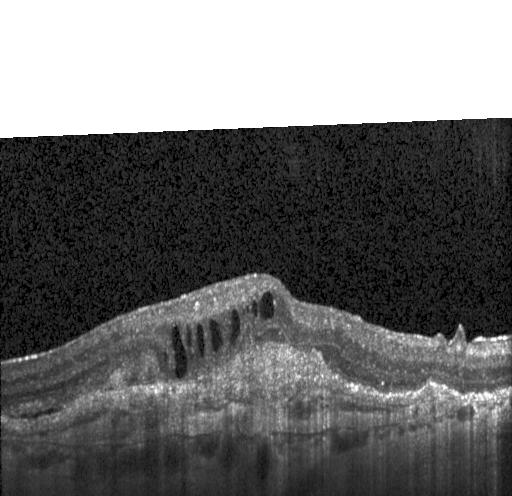
Dx: a choroidal neovascular membrane.